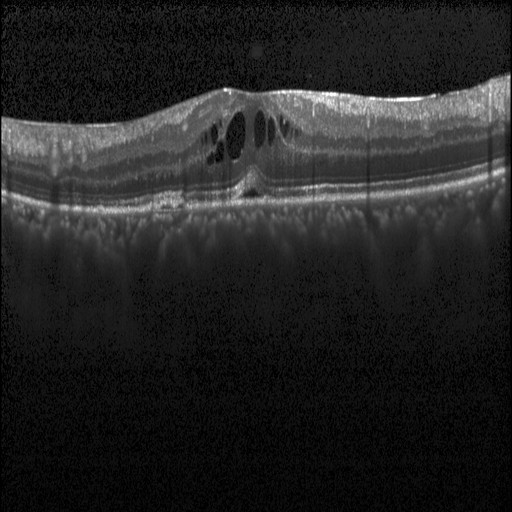
OCT scan showing DME.